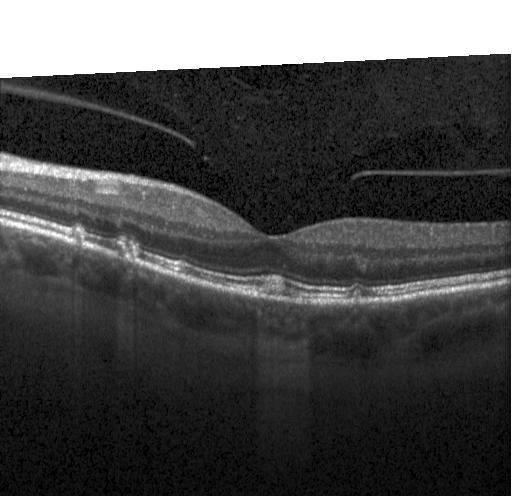
SD-OCT; instrument: Heidelberg Spectralis; retinal OCT cross-section.
Assessment: sub-RPE drusenoid deposits.